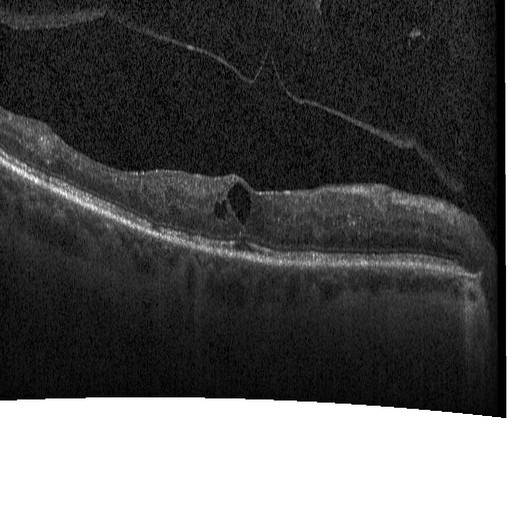 OCT line scan; horizontal scan through the fovea
Diagnosis: DME.